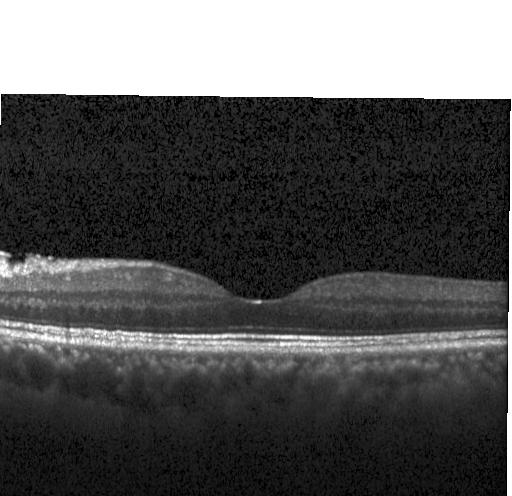 Acquired on a Heidelberg Spectralis. SD-OCT. Retinal OCT B-scan
OCT finding: neither CNV, DME, nor drusen.